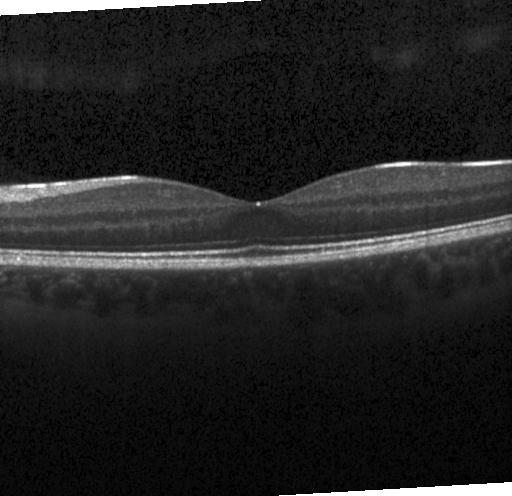 Acquired on a Heidelberg Spectralis · retinal OCT cross-section · spectral-domain optical coherence tomography.
Impression: no evidence of choroidal neovascularization, diabetic macular edema, or drusen.